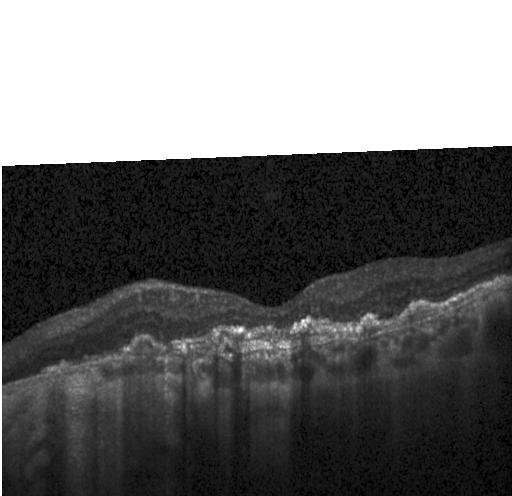 OCT scan showing a choroidal neovascular membrane.